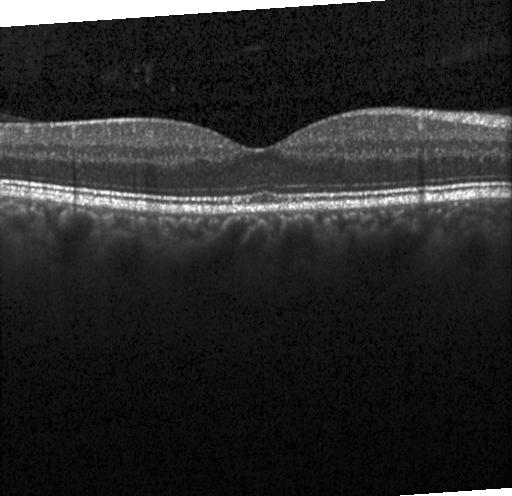 Diagnosis: no choroidal neovascularization, no diabetic macular edema, and no drusen.